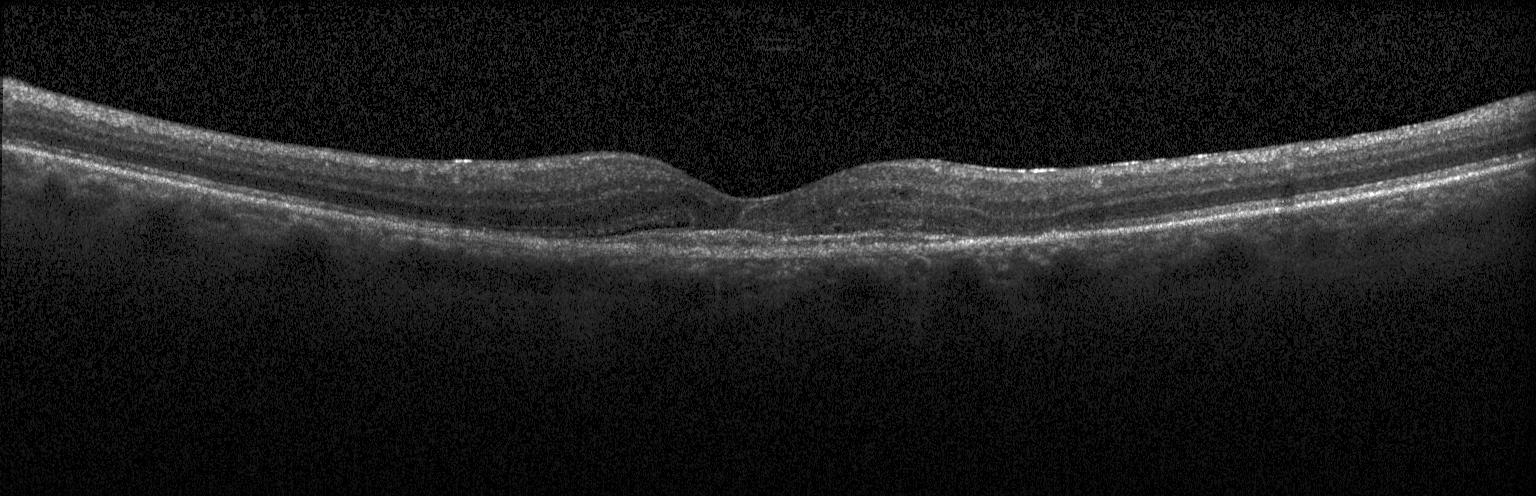
Macular OCT: a choroidal neovascular membrane.